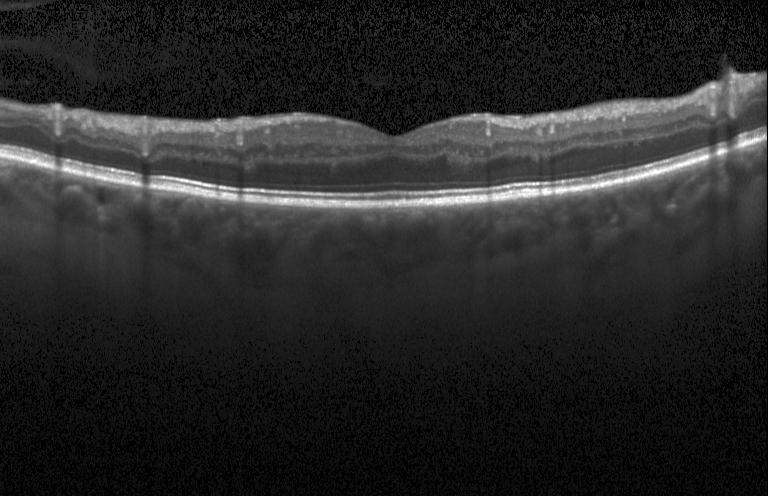
Impression: no evidence of CNV, DME, or drusen.